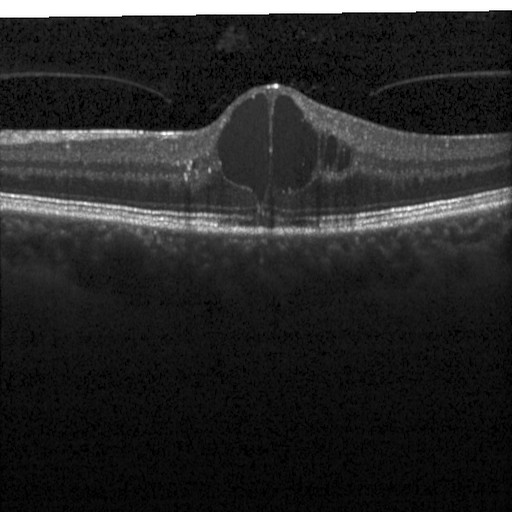

Heidelberg Spectralis; retinal OCT cross-section; macular scan
Dx: DME.